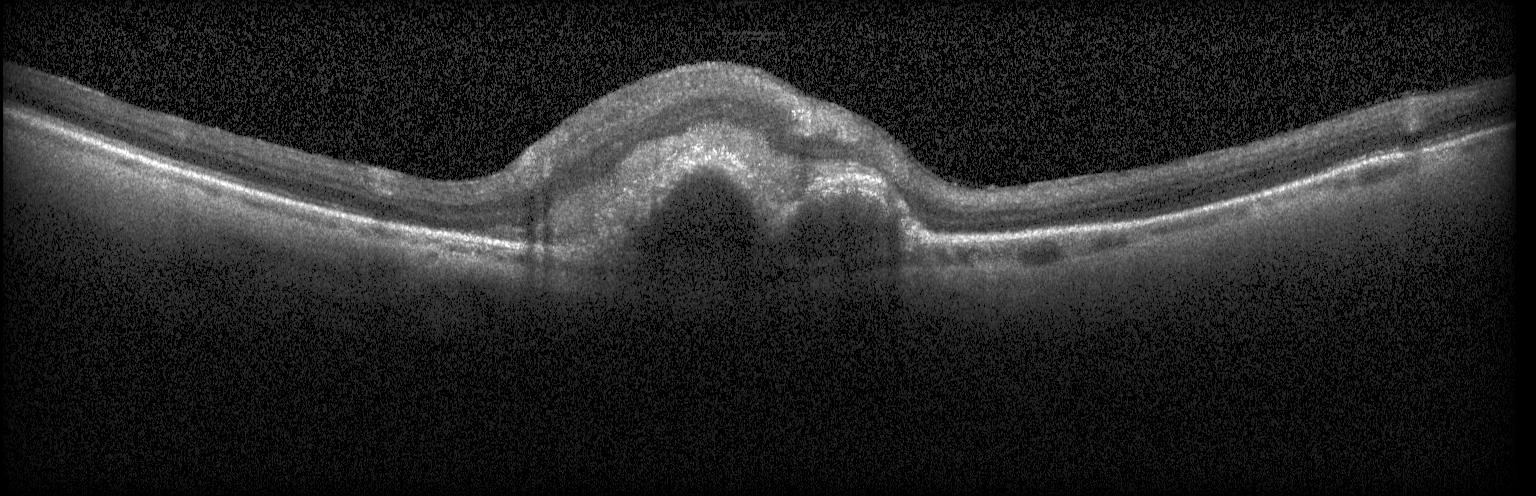 Finding: a choroidal neovascular membrane.